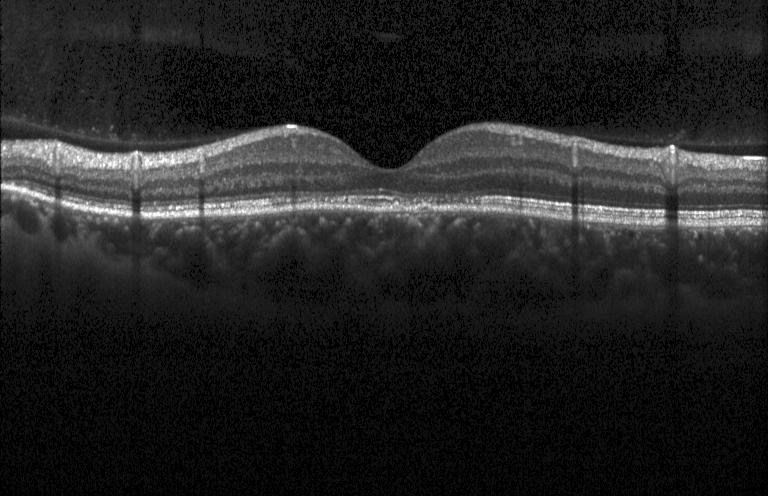

Through the macula; OCT B-scan; spectral-domain optical coherence tomography.
Finding: no choroidal neovascularization, diabetic macular edema, or drusen.